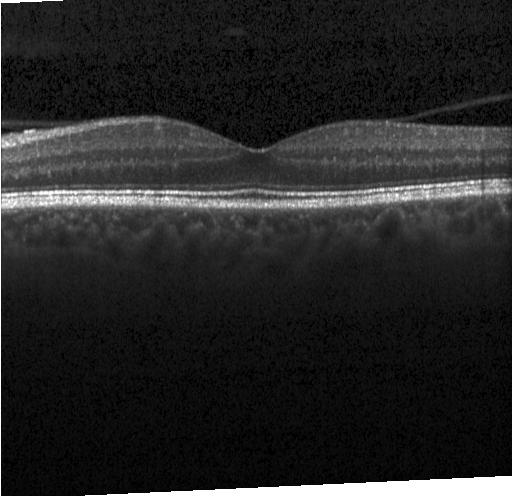
OCT B-scan — Finding: no evidence of choroidal neovascularization, diabetic macular edema, or drusen.